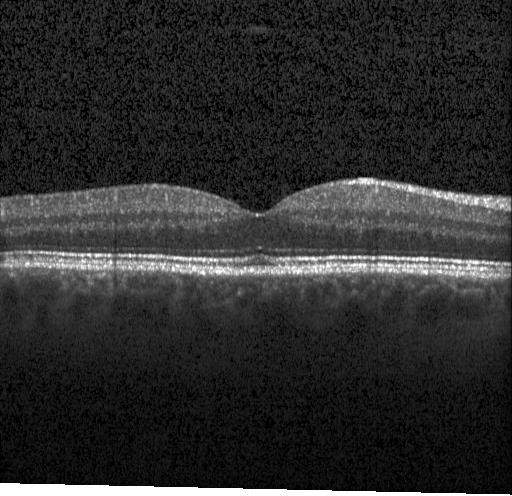
Impression: no choroidal neovascularization, no diabetic macular edema, and no drusen.